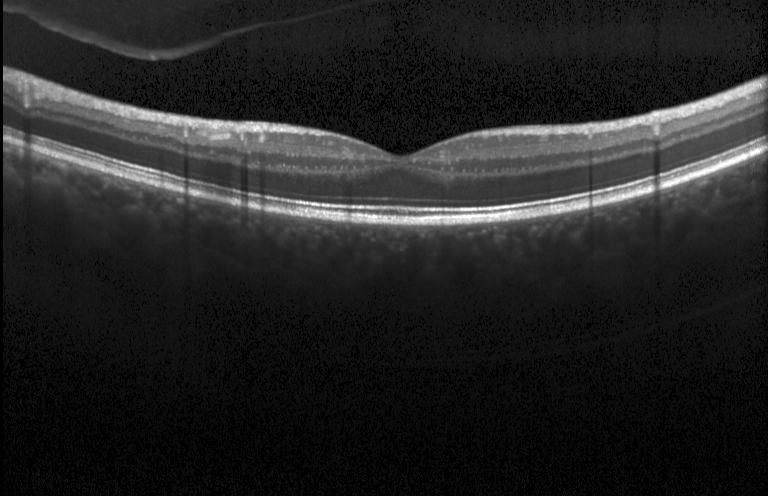
Horizontal scan through the fovea, OCT line scan, instrument: Heidelberg Spectralis, SD-OCT. Macular OCT: neither CNV, DME, nor drusen.